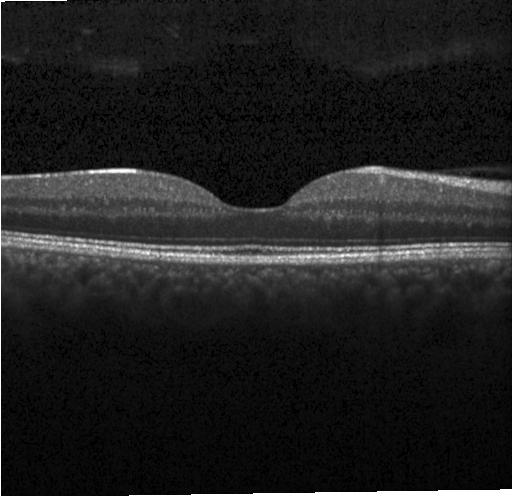
OCT line scan · fovea-centered.
Impression: no evidence of choroidal neovascularization, diabetic macular edema, or drusen.